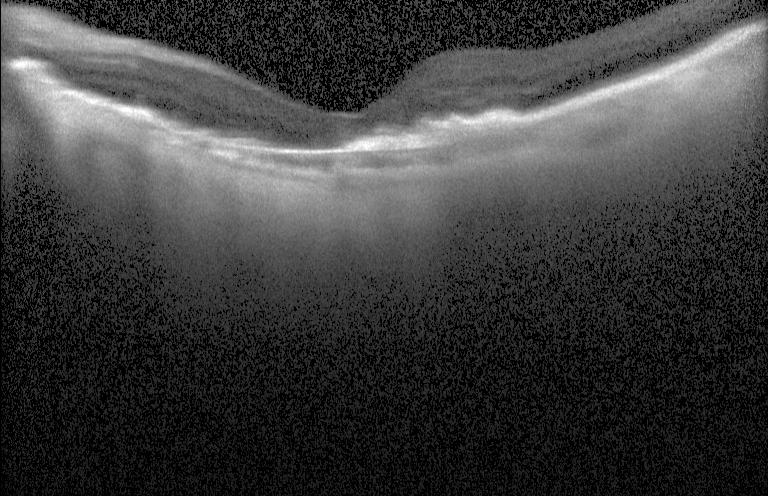 OCT finding: a choroidal neovascular membrane.